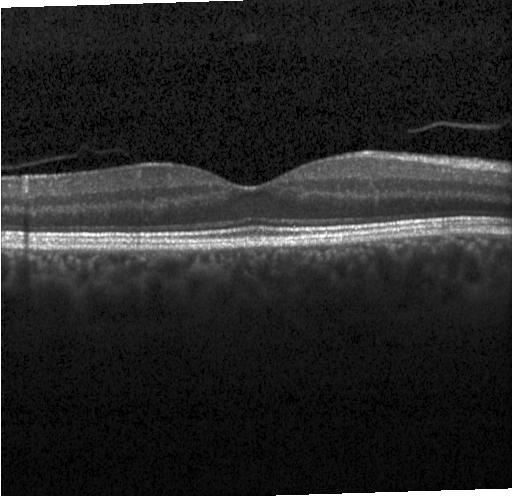

Retinal OCT B-scan. Instrument: Heidelberg Spectralis.
Macular OCT: neither CNV, DME, nor drusen.